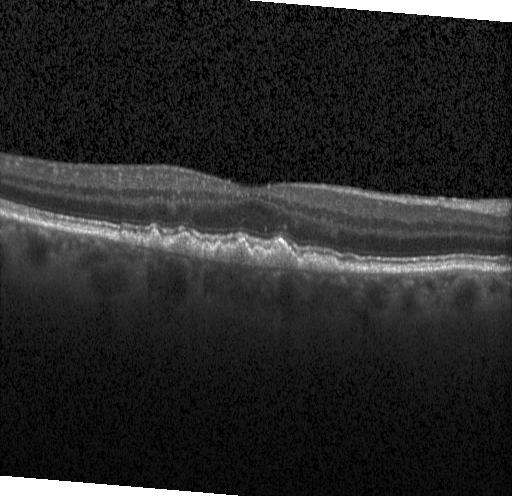
SD-OCT · Heidelberg Spectralis · OCT line scan · horizontal scan through the fovea. Finding: drusen.